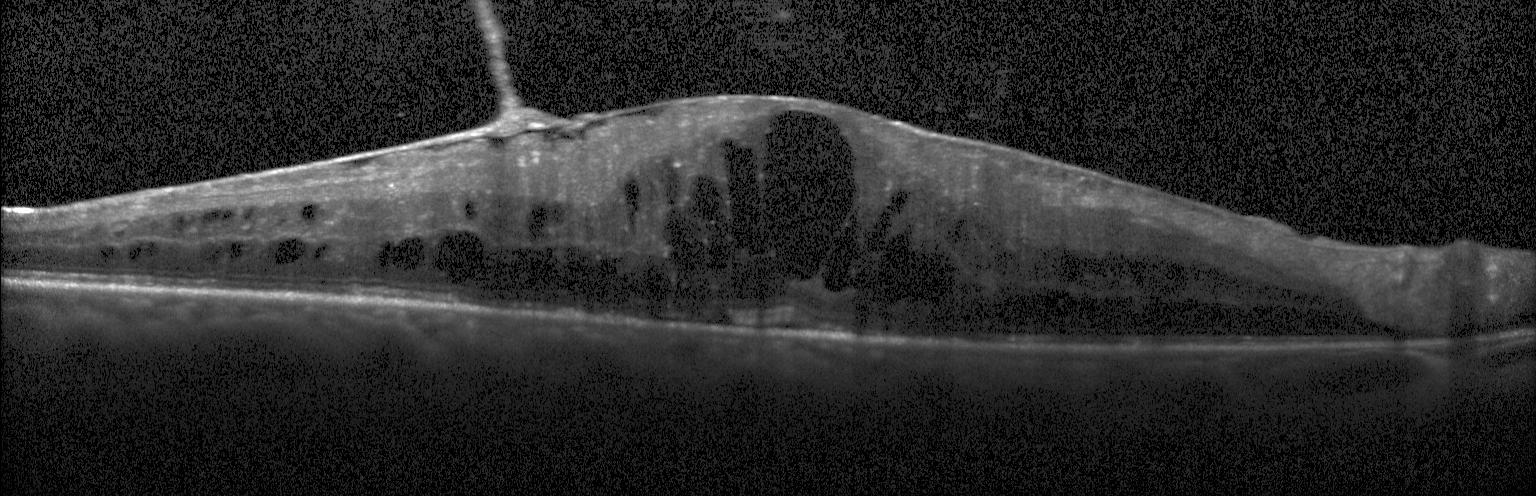

Diagnosis: DME.